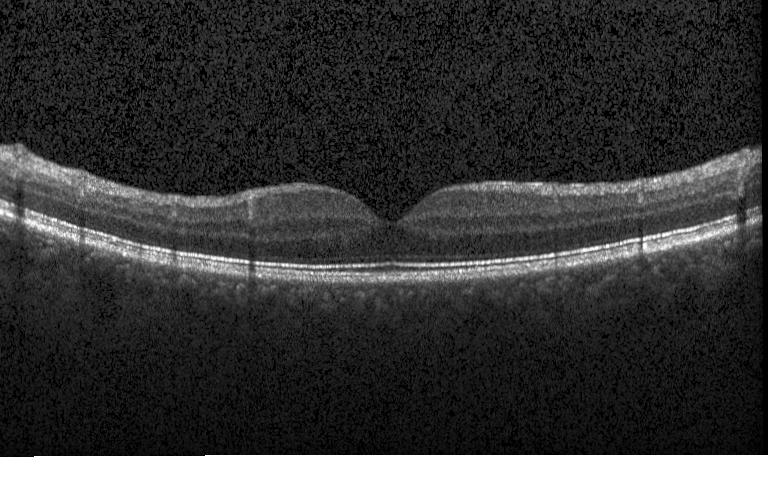

Instrument: Heidelberg Spectralis · through the macula · optical coherence tomography B-scan · spectral-domain OCT — Neither choroidal neovascularization, diabetic macular edema, nor drusen.